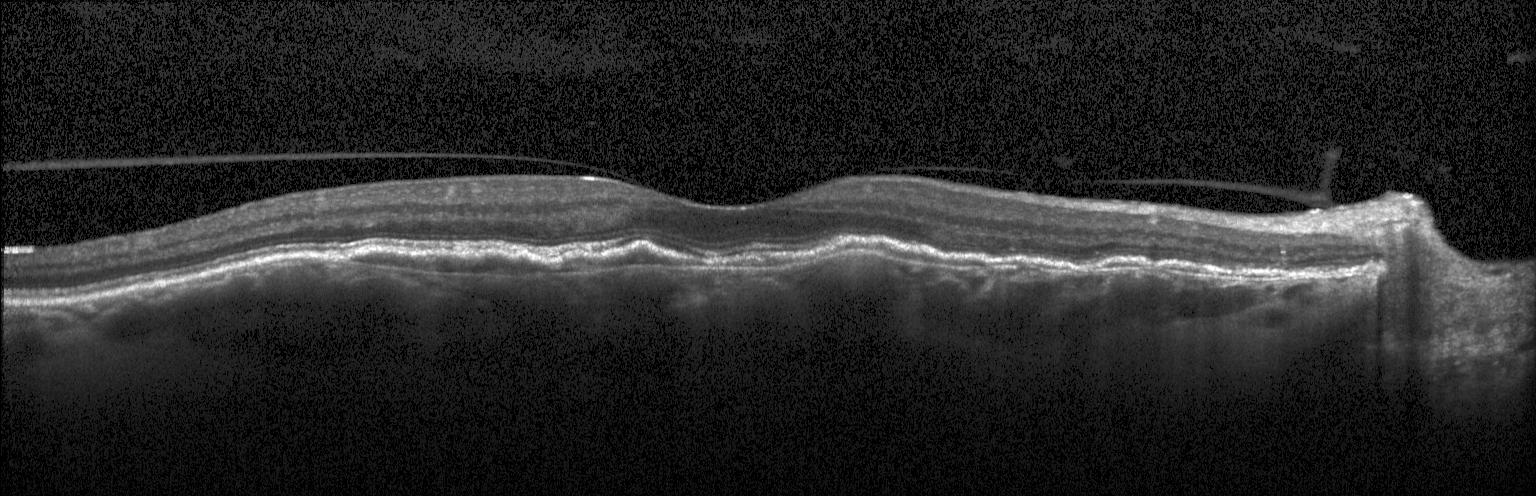 Diagnosis: a choroidal neovascular membrane.